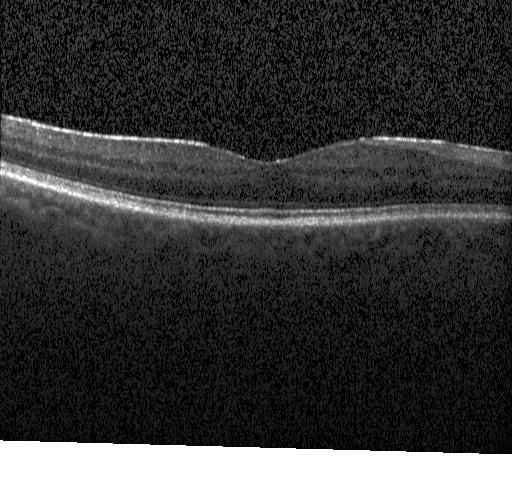 Macular OCT demonstrating no choroidal neovascularization, no diabetic macular edema, and no drusen.